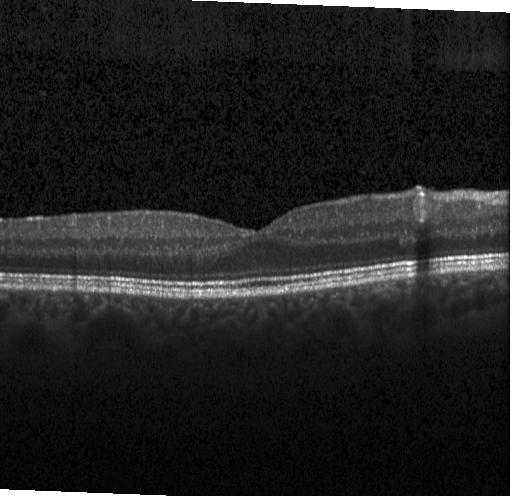 The scan shows no choroidal neovascularization, no diabetic macular edema, and no drusen.